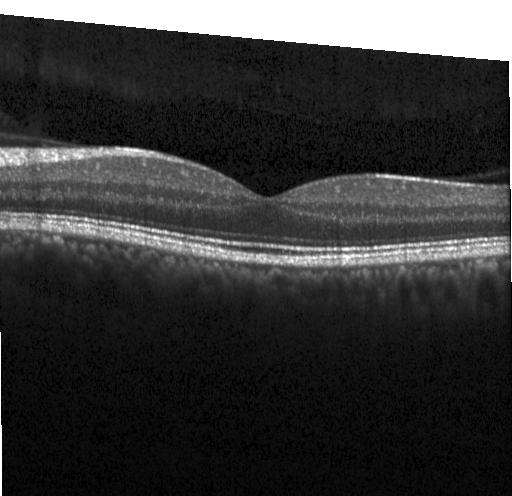 Retinal OCT cross-section — Finding: neither choroidal neovascularization, diabetic macular edema, nor drusen.